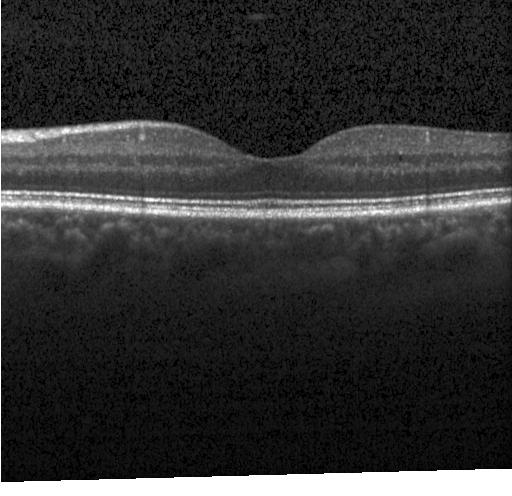 Diagnosis: no choroidal neovascularization, diabetic macular edema, or drusen.